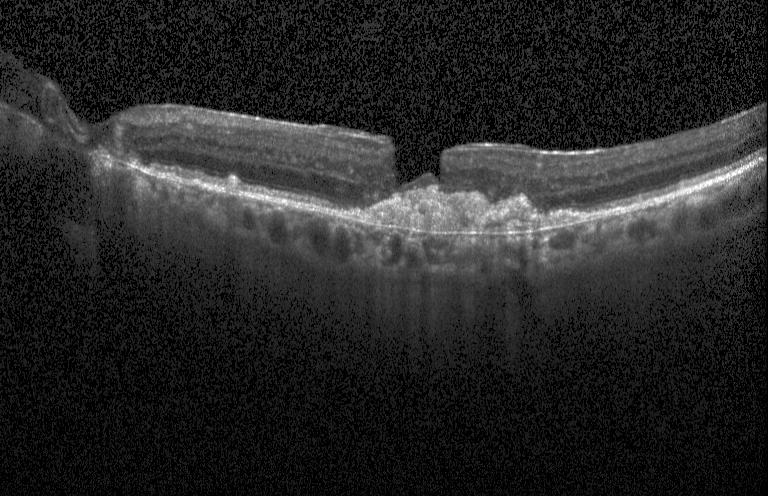

Optical coherence tomography B-scan · macular scan.
Assessment: CNV.